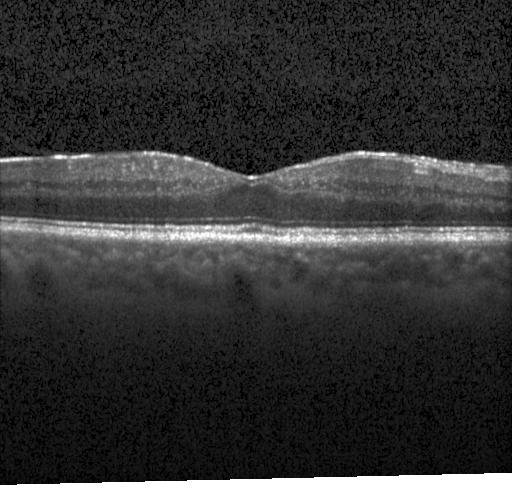 Heidelberg Spectralis. Macular scan. Spectral-domain OCT. Retinal OCT cross-section.
This B-scan demonstrates neither CNV, DME, nor drusen.